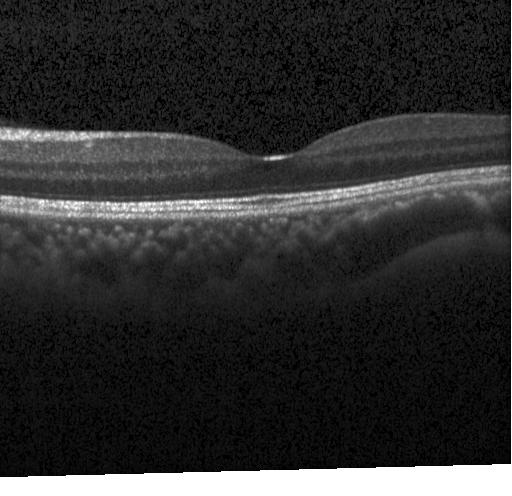

Retinal OCT B-scan; instrument: Heidelberg Spectralis; spectral-domain optical coherence tomography — Impression: no choroidal neovascularization, diabetic macular edema, or drusen.